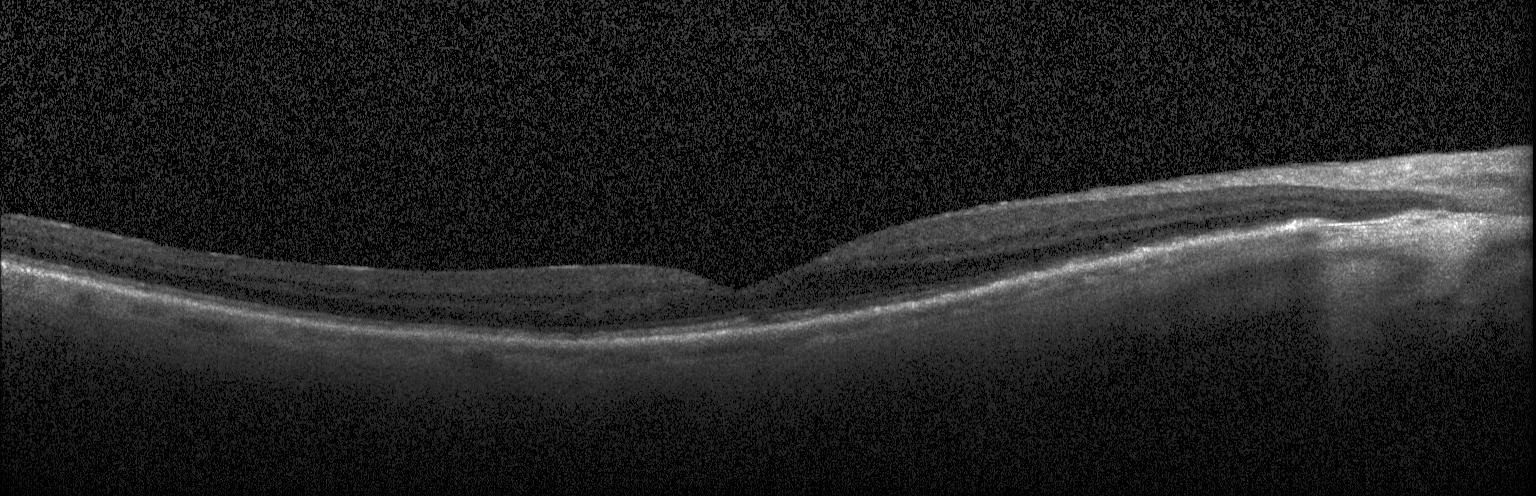 Diagnosis: no evidence of choroidal neovascularization, diabetic macular edema, or drusen.